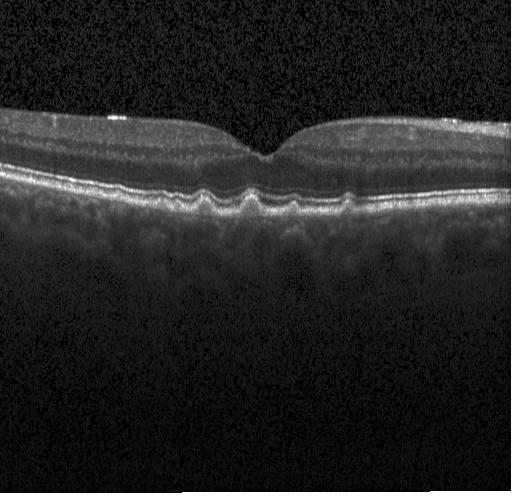

OCT line scan
Finding: drusen.